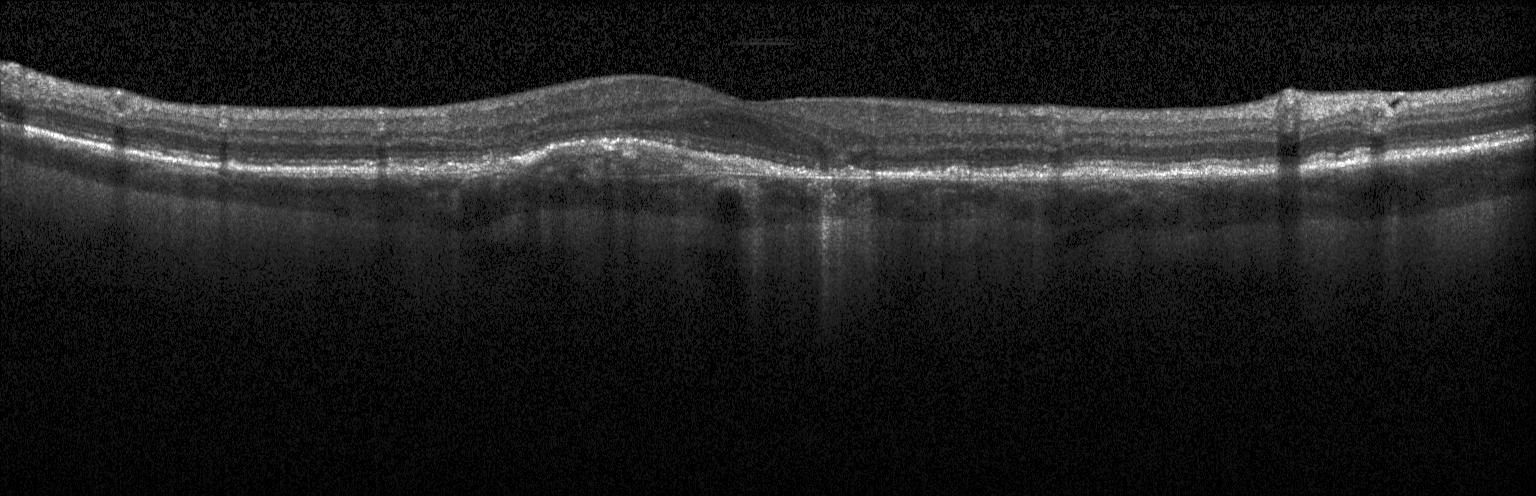 Retinal OCT cross-section showing a choroidal neovascular membrane.